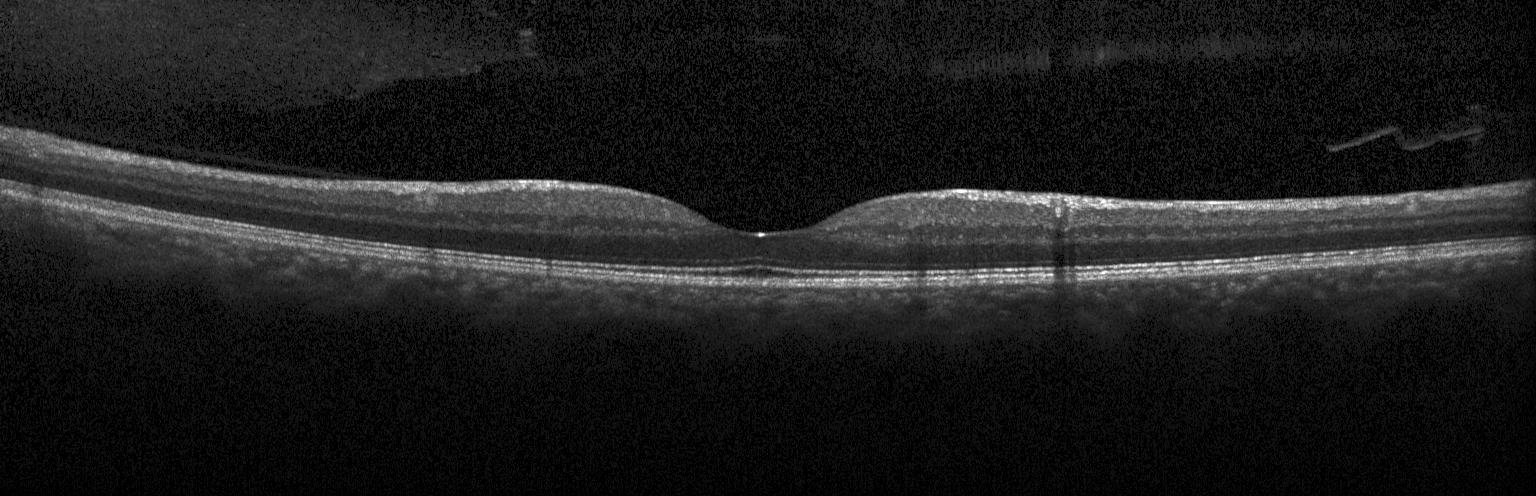
Retinal OCT B-scan.
No evidence of choroidal neovascularization, diabetic macular edema, or drusen.